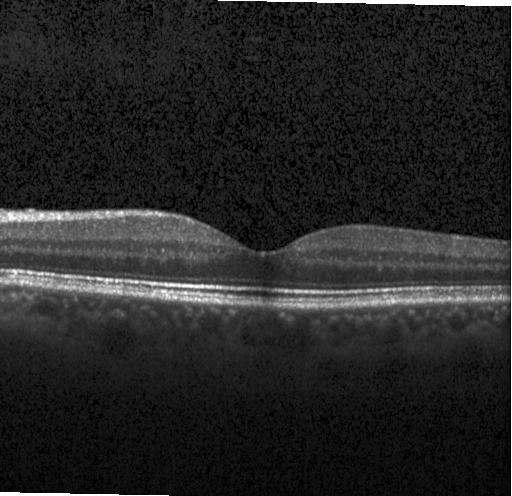 Dx: no evidence of CNV, DME, or drusen.